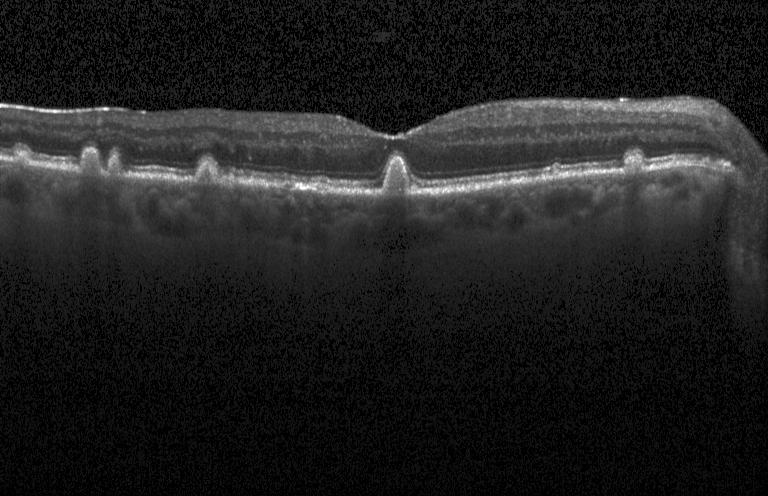
Heidelberg Spectralis OCT system. SD-OCT. Optical coherence tomography B-scan
Diagnosis: drusen.